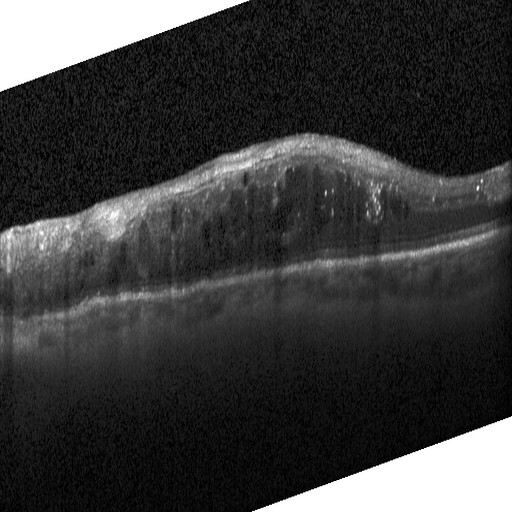
SD-OCT, fovea-centered, OCT B-scan — Dx: DME.